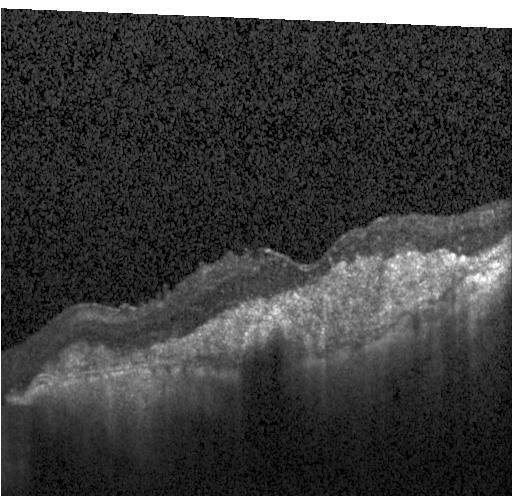
Optical coherence tomography scan · spectral-domain optical coherence tomography · Heidelberg Spectralis OCT system — Impression: a choroidal neovascular membrane.